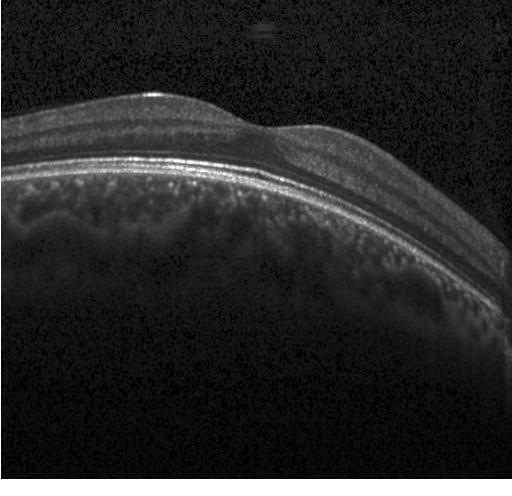
This B-scan demonstrates no choroidal neovascularization, diabetic macular edema, or drusen.